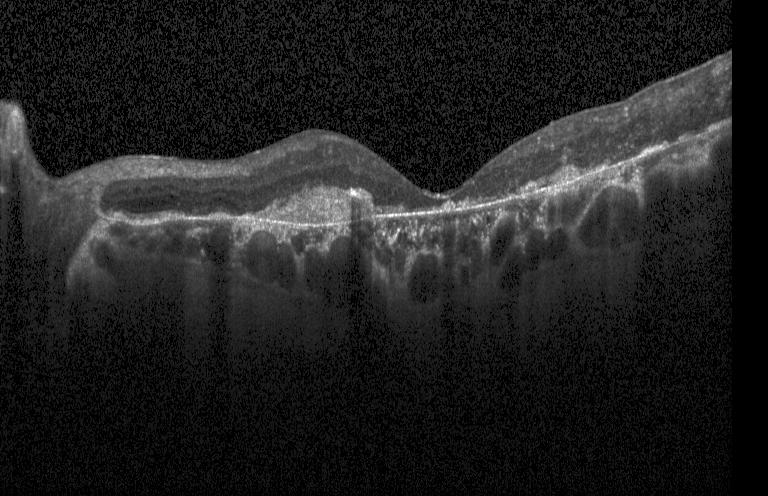 Centered on the fovea, retinal OCT B-scan, Heidelberg Spectralis OCT system.
A choroidal neovascular membrane.